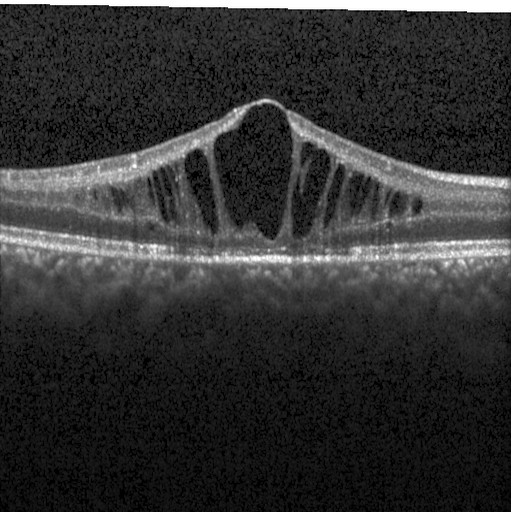 OCT B-scan.
Diabetic macular edema.